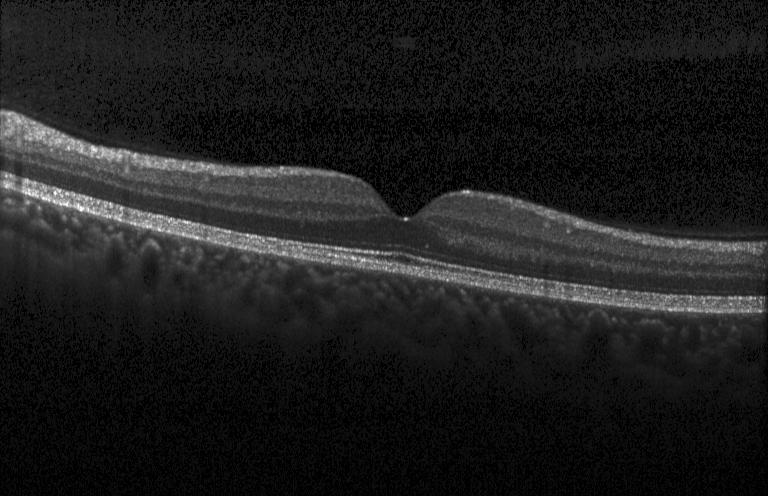
Retinal OCT B-scan
Impression: no evidence of choroidal neovascularization, diabetic macular edema, or drusen.